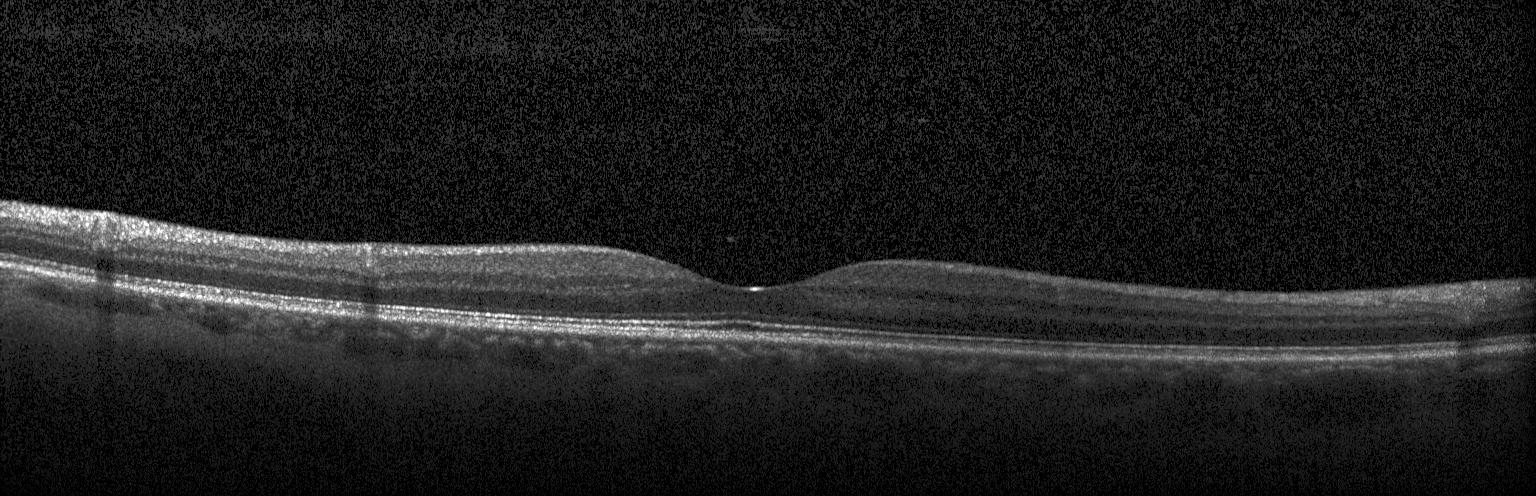

Retinal OCT cross-section showing no choroidal neovascularization, no diabetic macular edema, and no drusen.